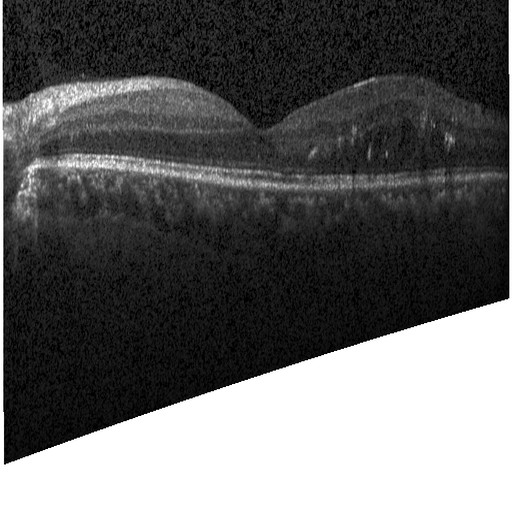

Optical coherence tomography B-scan; spectral-domain OCT; instrument: Heidelberg Spectralis.
OCT finding: diabetic macular edema.